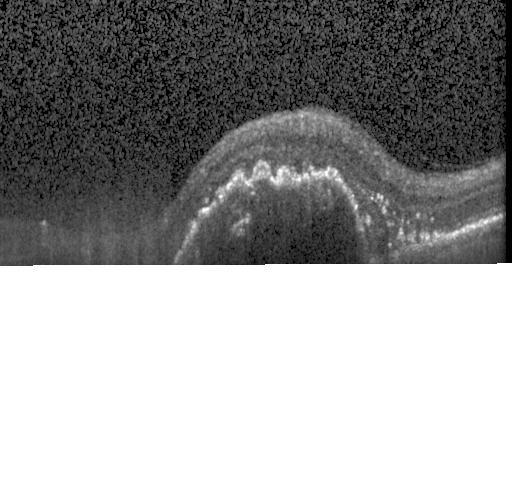

Optical coherence tomography scan, Heidelberg Spectralis, horizontal scan through the fovea, SD-OCT — The scan shows CNV.